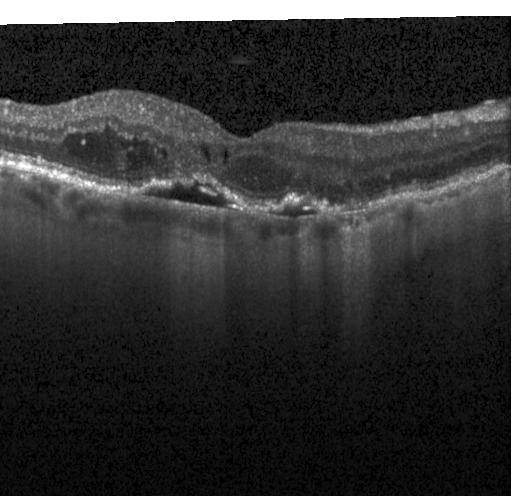 Retinal OCT cross-section, spectral-domain optical coherence tomography — OCT finding: CNV.